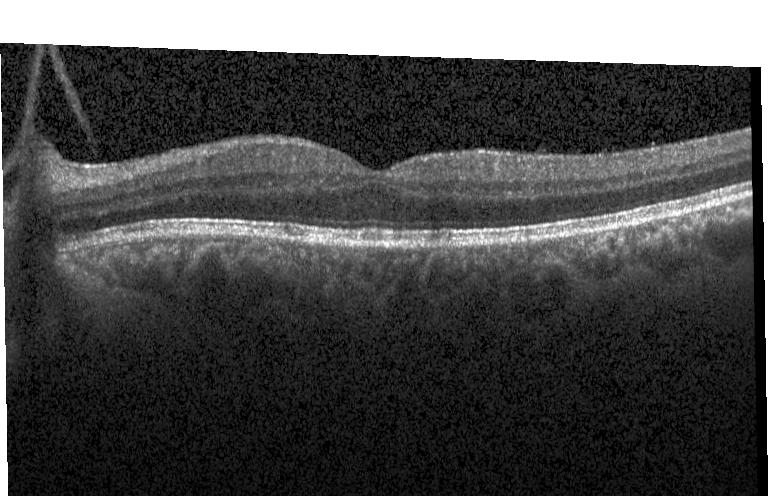 Dx: neither choroidal neovascularization, diabetic macular edema, nor drusen.